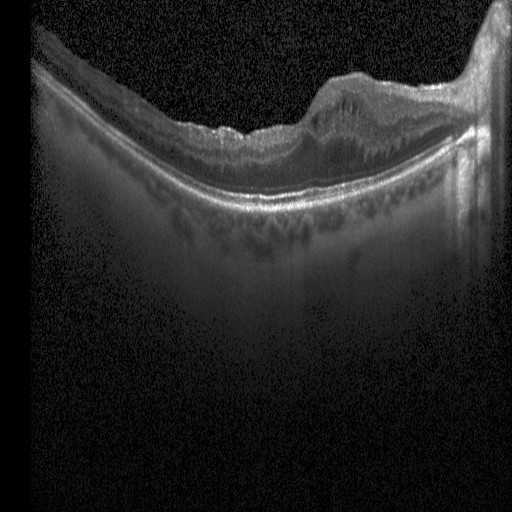 Acquired on a Heidelberg Spectralis, OCT line scan, centered on the fovea — Impression: diabetic macular edema (DME).